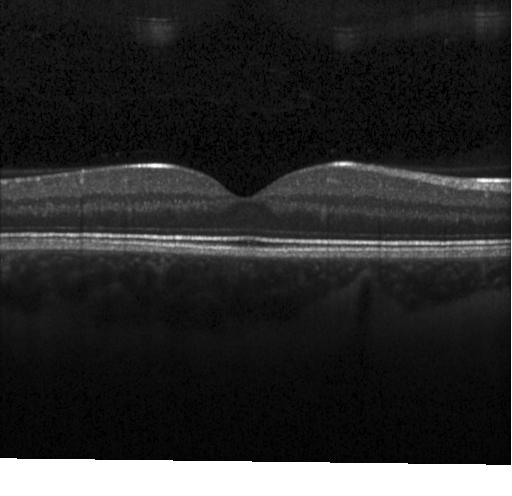 Finding: no CNV, no DME, and no drusen.